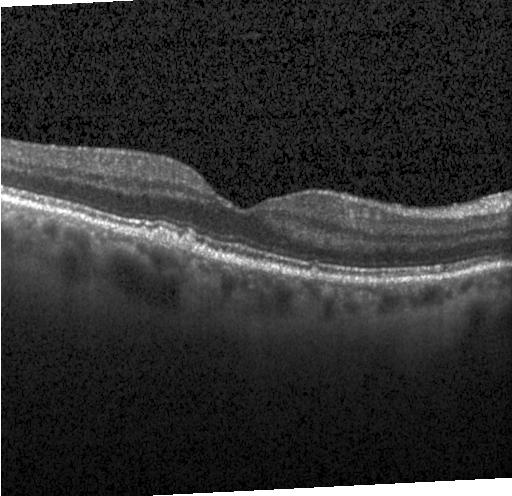

OCT line scan; acquired on a Heidelberg Spectralis — Assessment: drusen.